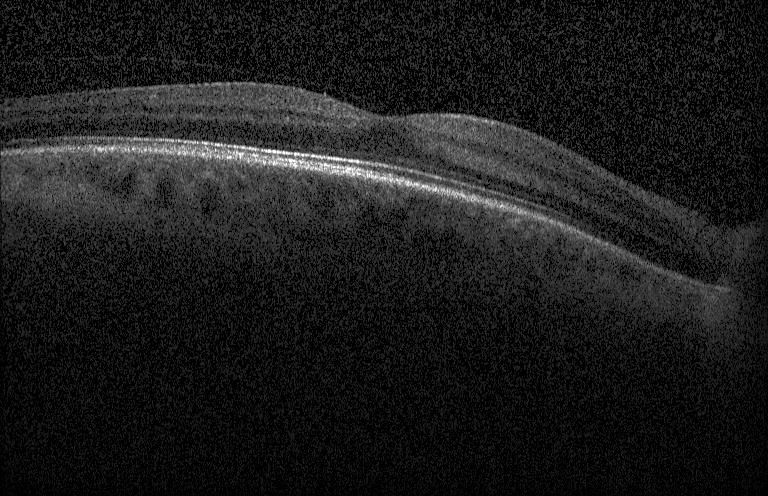 No evidence of CNV, DME, or drusen.